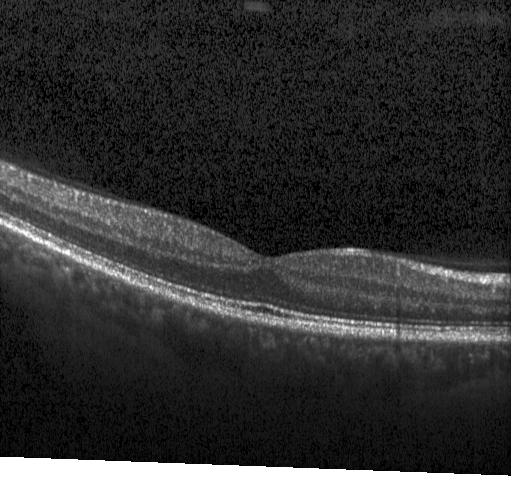
SD-OCT · optical coherence tomography B-scan · acquired on a Heidelberg Spectralis · fovea-centered — Diagnosis: no choroidal neovascularization, diabetic macular edema, or drusen.